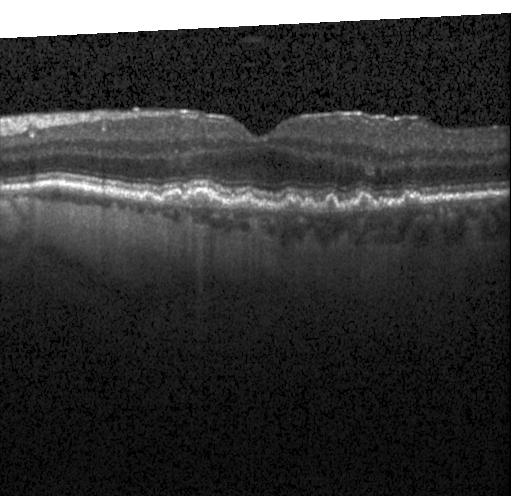 Heidelberg Spectralis; optical coherence tomography B-scan; spectral-domain OCT
This B-scan demonstrates multiple drusen.